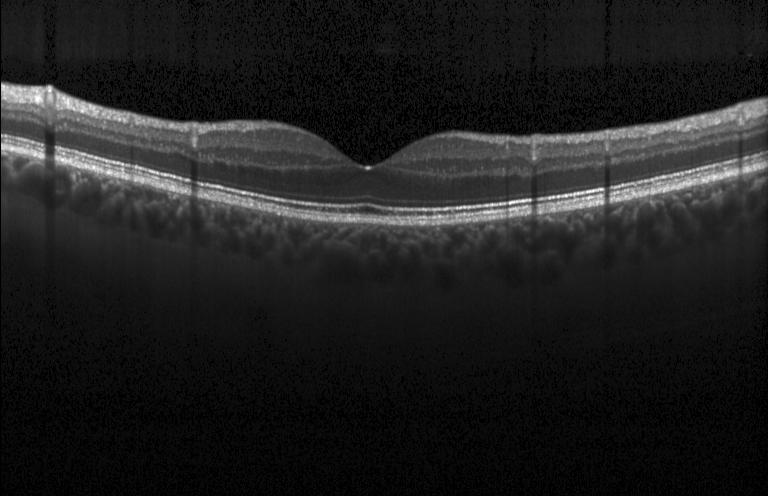 Centered on the fovea; acquired on a Heidelberg Spectralis; spectral-domain optical coherence tomography; retinal OCT B-scan
Dx: no choroidal neovascularization, no diabetic macular edema, and no drusen.